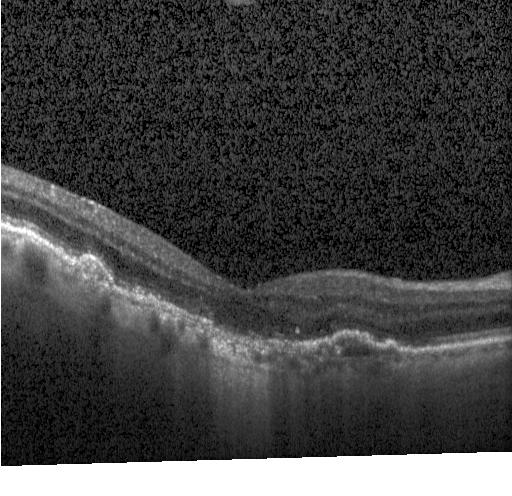

Spectral-domain optical coherence tomography, retinal OCT B-scan, centered on the fovea, acquired on a Heidelberg Spectralis.
Macular OCT: a choroidal neovascular membrane.